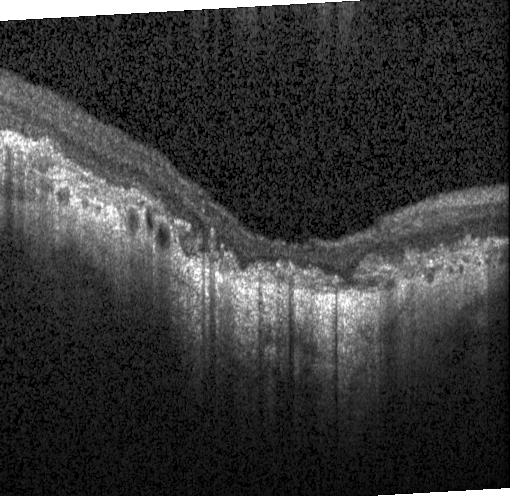 Retinal OCT cross-section · centered on the fovea · spectral-domain optical coherence tomography — Dx: choroidal neovascularization (CNV).